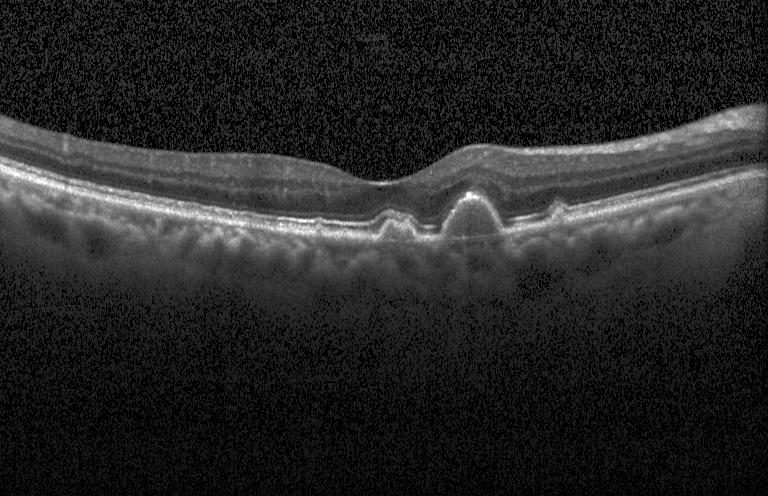

Horizontal scan through the fovea. SD-OCT. OCT line scan.
The scan shows sub-RPE drusenoid deposits.